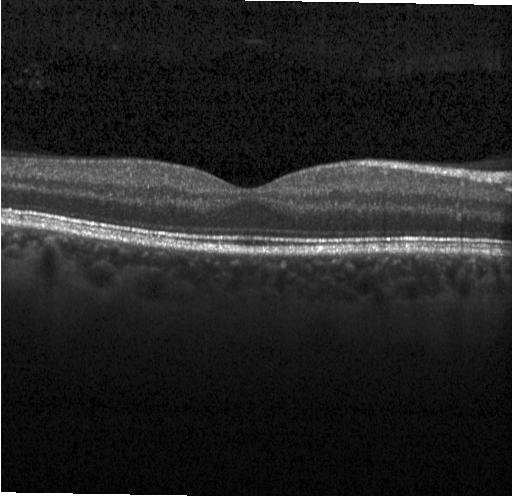 Optical coherence tomography scan. Impression: no evidence of choroidal neovascularization, diabetic macular edema, or drusen.